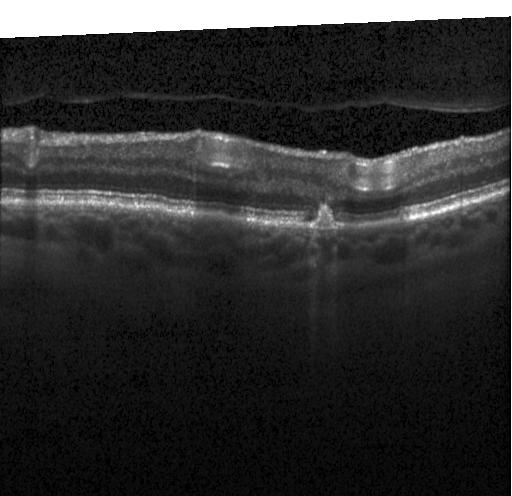

Optical coherence tomography scan.
Diagnosis: drusen.